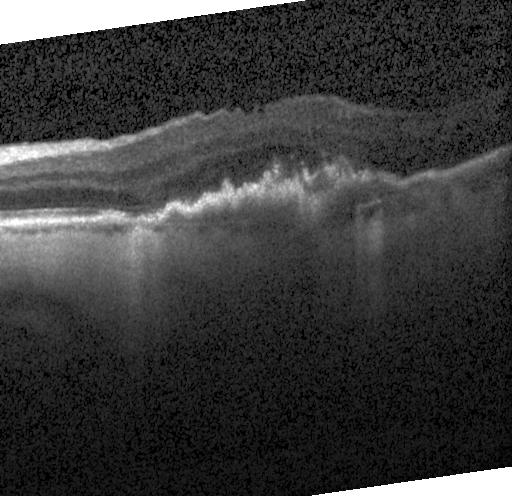 Impression: CNV.